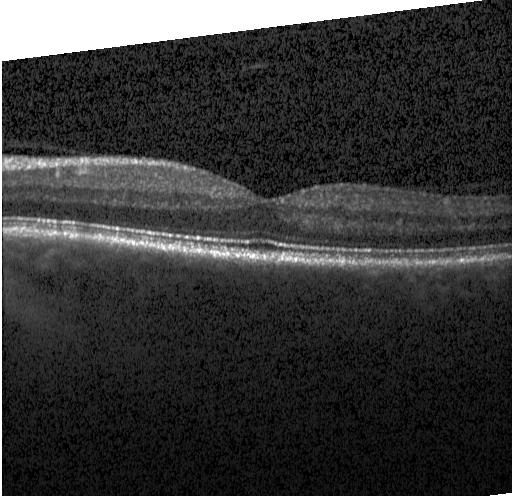
Acquired on a Heidelberg Spectralis, optical coherence tomography B-scan.
Finding: neither choroidal neovascularization, diabetic macular edema, nor drusen.